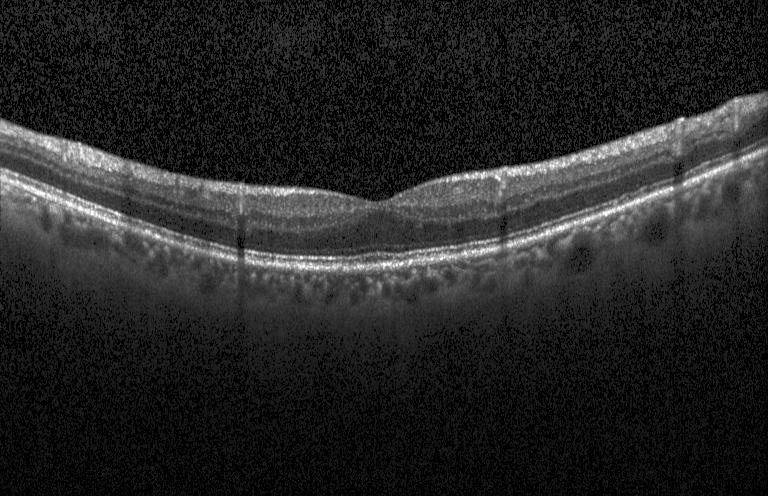
Optical coherence tomography scan, Heidelberg Spectralis OCT system.
Assessment: neither choroidal neovascularization, diabetic macular edema, nor drusen.